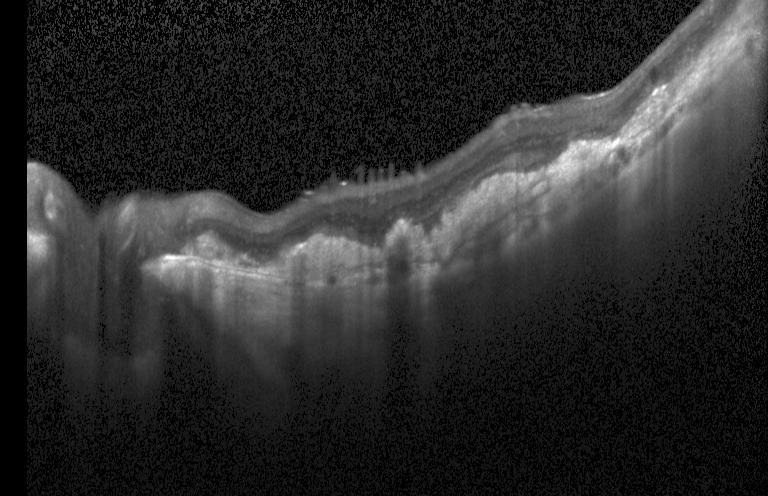
Retinal OCT cross-section. Macular OCT: choroidal neovascularization.